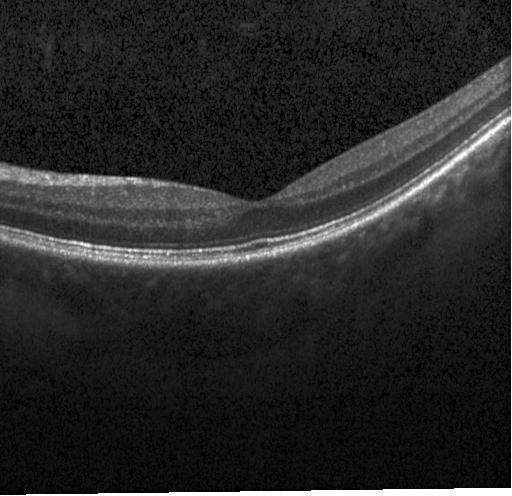
Optical coherence tomography B-scan. Heidelberg Spectralis OCT system. Spectral-domain OCT. Horizontal scan through the fovea. Finding: no evidence of choroidal neovascularization, diabetic macular edema, or drusen.